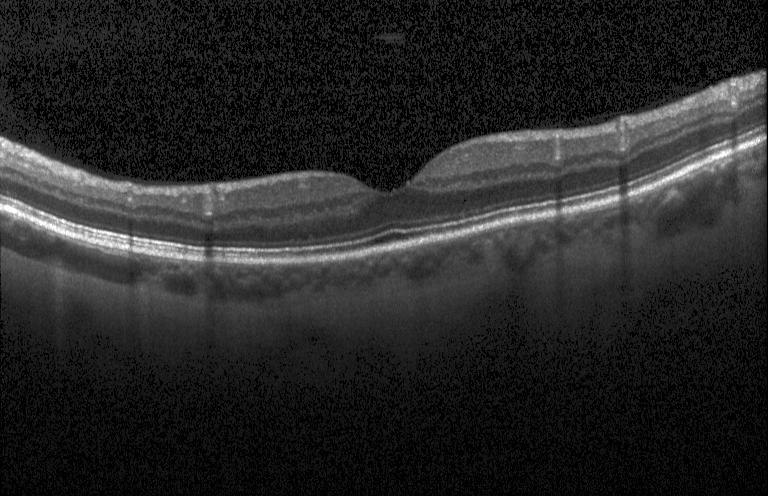
Macular scan; SD-OCT; optical coherence tomography B-scan. Finding: no choroidal neovascularization, diabetic macular edema, or drusen.